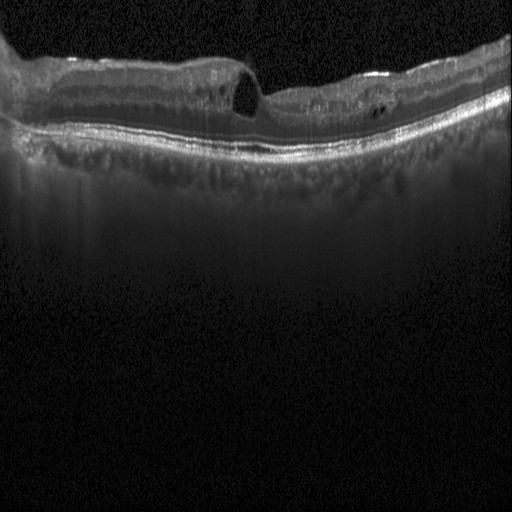
Horizontal scan through the fovea · optical coherence tomography scan
This B-scan demonstrates diabetic macular edema.